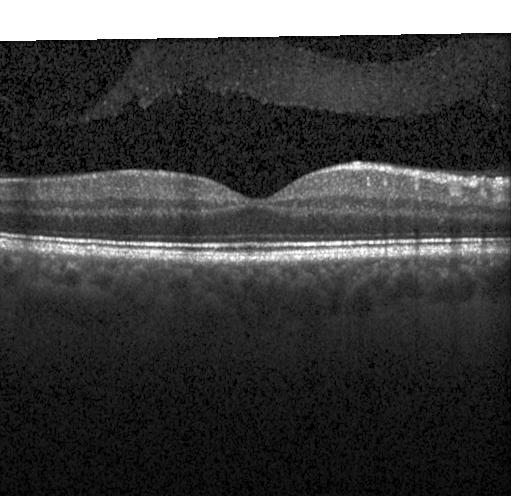 Diagnosis: no evidence of CNV, DME, or drusen.